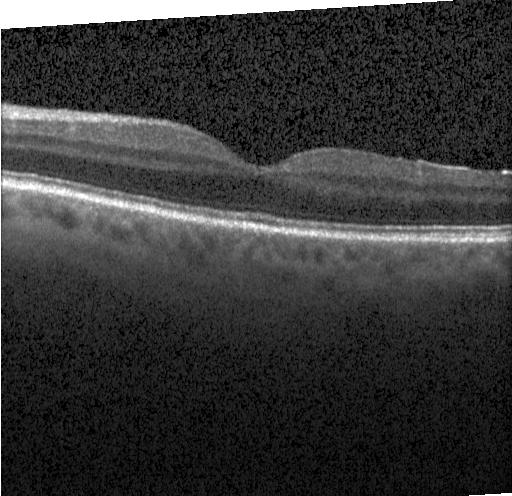

Retinal OCT cross-section showing no choroidal neovascularization, no diabetic macular edema, and no drusen.